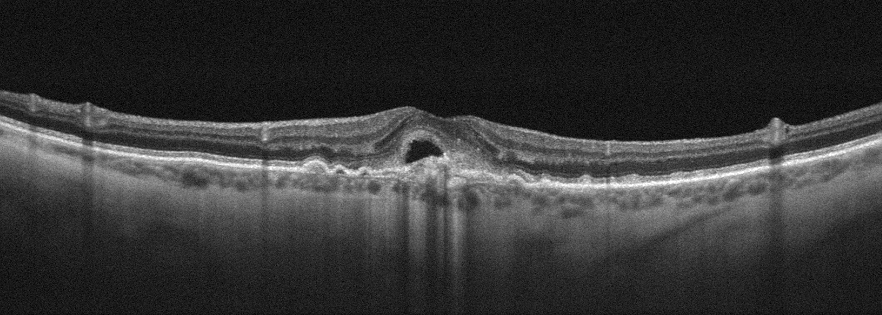
OD, retinal OCT cross-section. Finding: age-related macular degeneration (AMD).